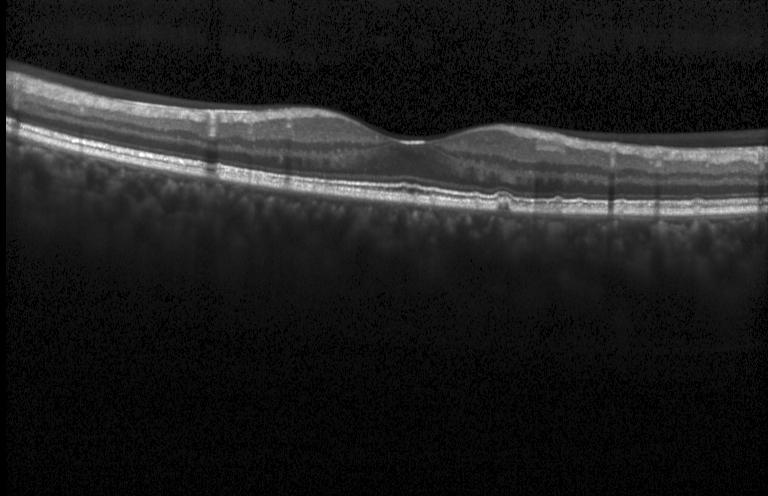 Diagnosis: drusen.